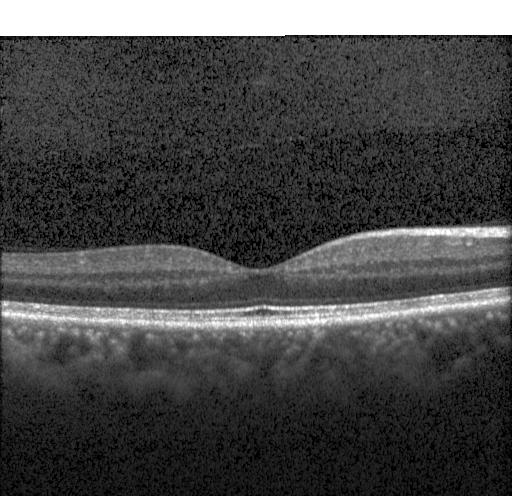

Spectral-domain optical coherence tomography · optical coherence tomography scan · macular scan · Heidelberg Spectralis
The scan shows no choroidal neovascularization, no diabetic macular edema, and no drusen.